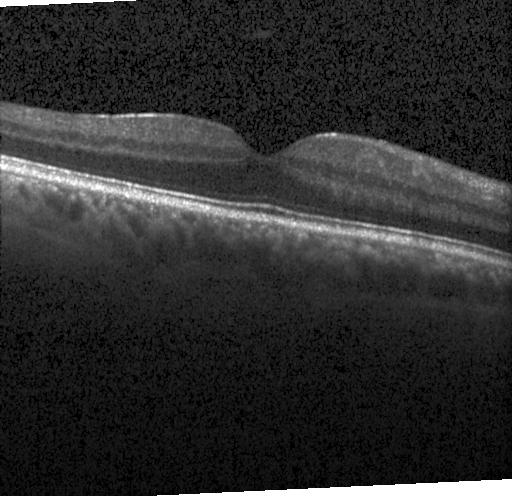
Optical coherence tomography scan
Macular OCT: no evidence of choroidal neovascularization, diabetic macular edema, or drusen.